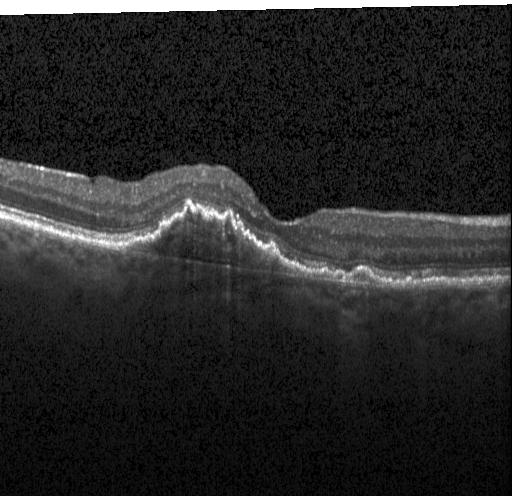

Heidelberg Spectralis OCT system. Retinal OCT B-scan. Macular scan. Spectral-domain optical coherence tomography
Dx: choroidal neovascularization.